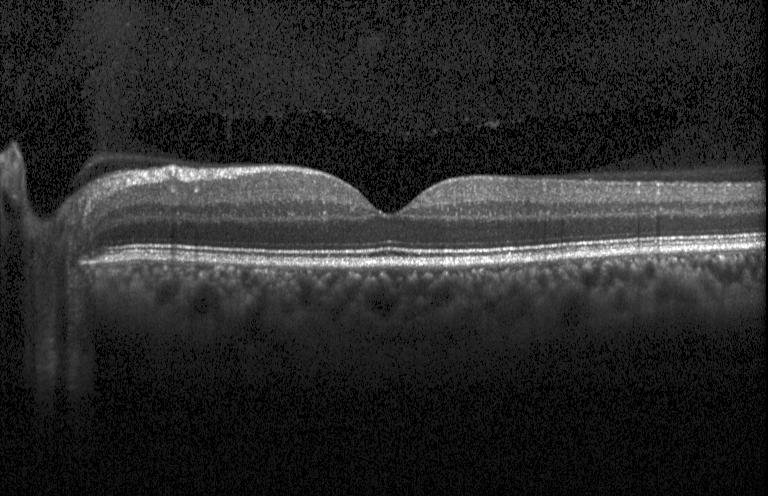

OCT line scan. Dx: neither CNV, DME, nor drusen.